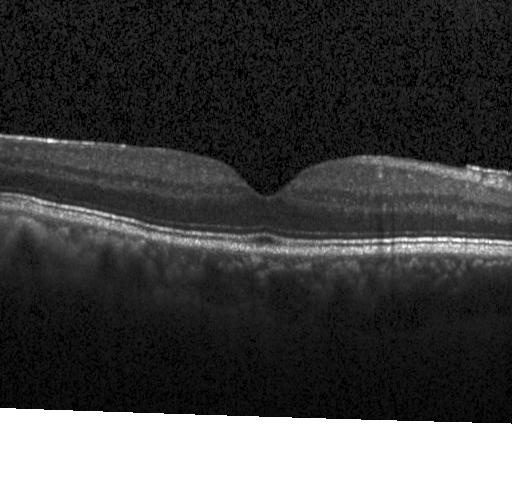
Assessment: no evidence of choroidal neovascularization, diabetic macular edema, or drusen.